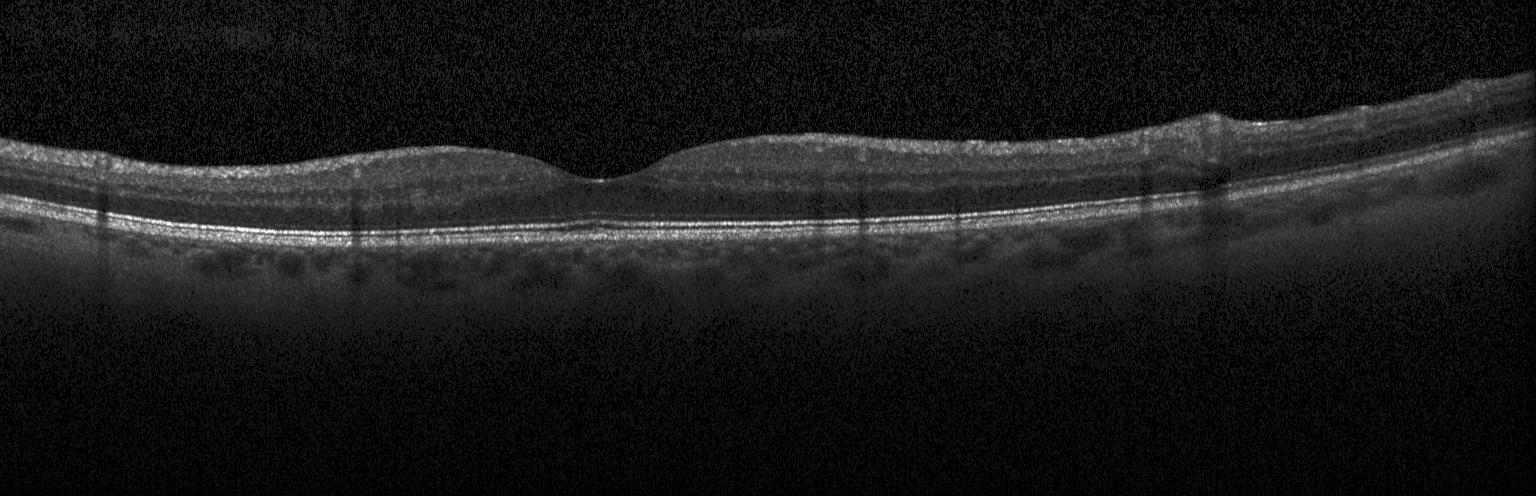
This B-scan demonstrates no CNV, no DME, and no drusen.